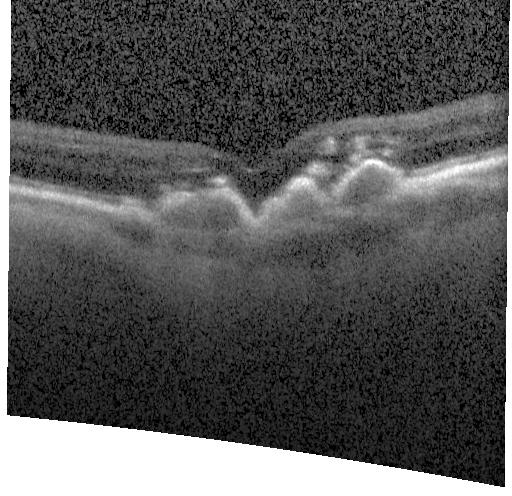
OCT line scan. SD-OCT. Heidelberg Spectralis OCT system
Finding: choroidal neovascularization (CNV).